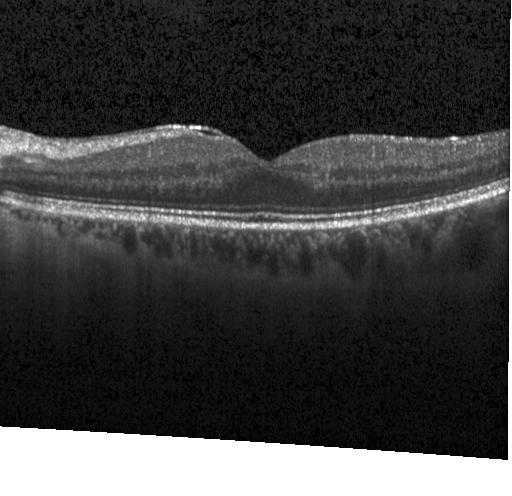 This B-scan demonstrates neither CNV, DME, nor drusen.